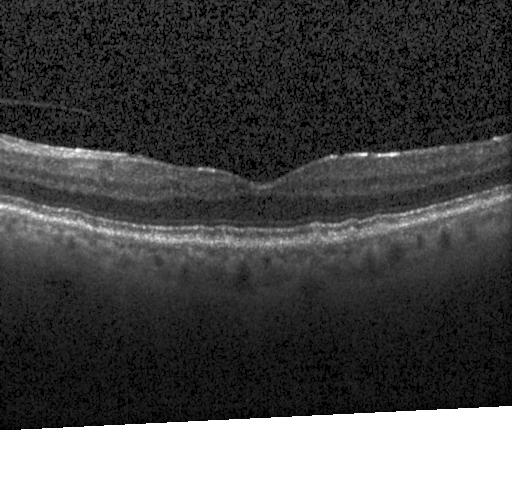
OCT B-scan showing drusen.